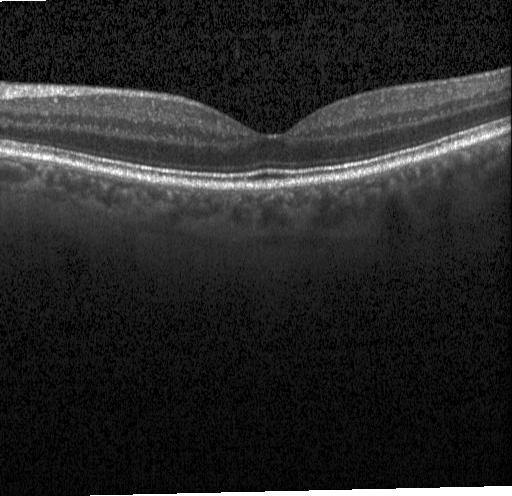
Impression: no evidence of choroidal neovascularization, diabetic macular edema, or drusen.